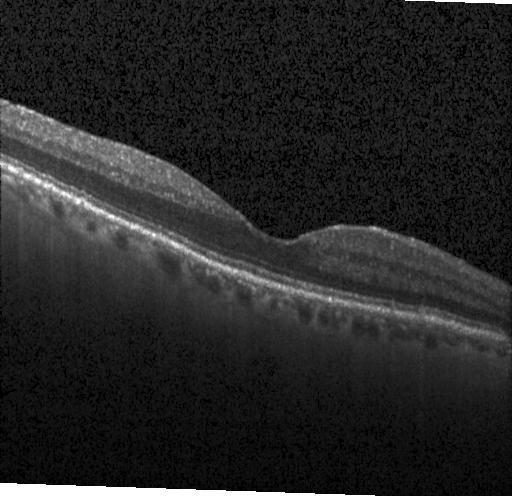
OCT line scan · spectral-domain OCT.
The scan shows neither CNV, DME, nor drusen.